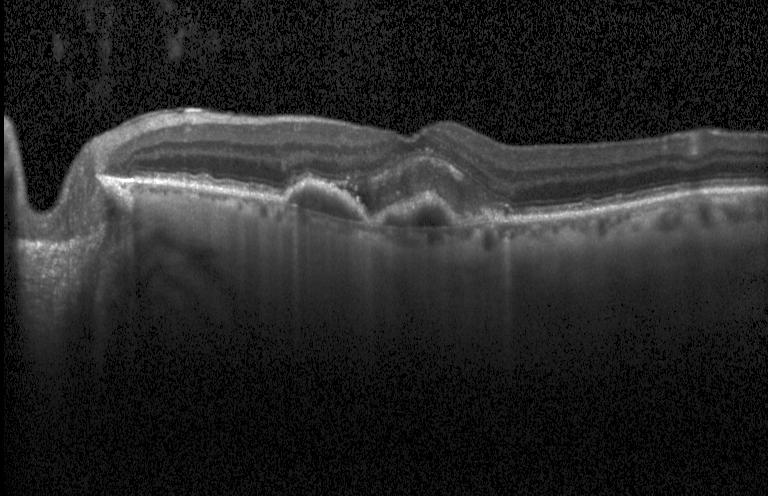

Choroidal neovascularization.